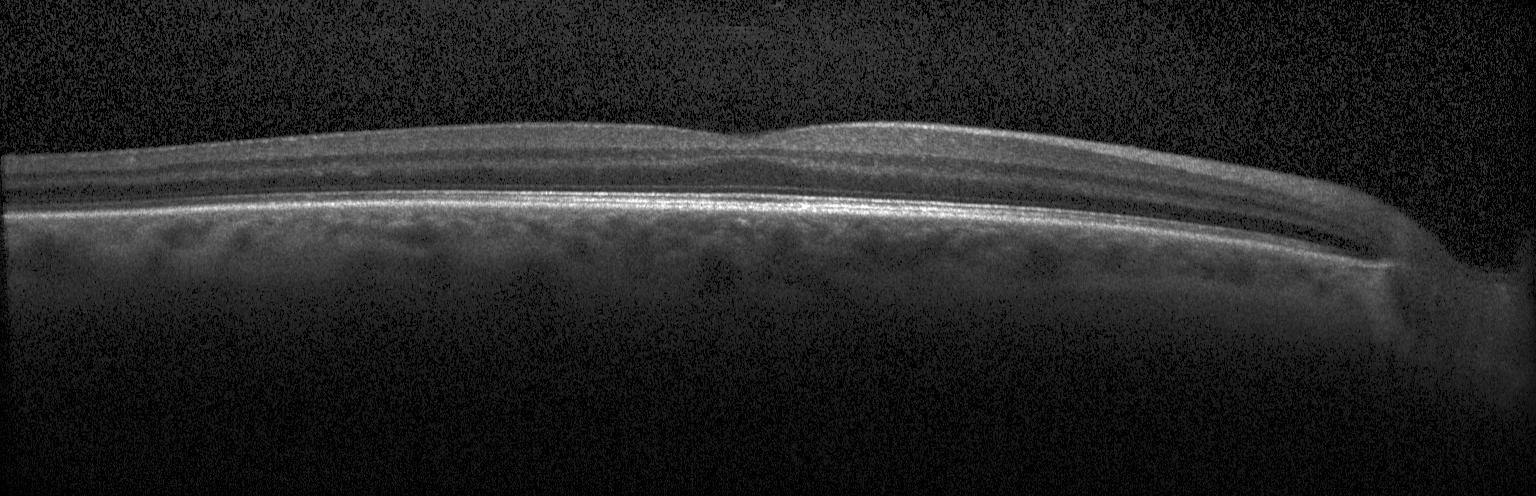

The scan shows no CNV, DME, or drusen.